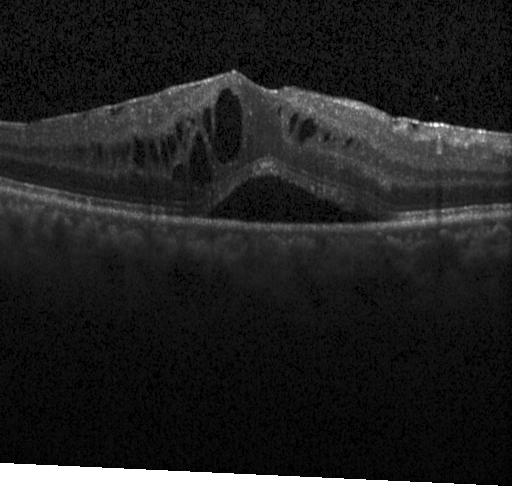
Dx: diabetic macular edema (DME).